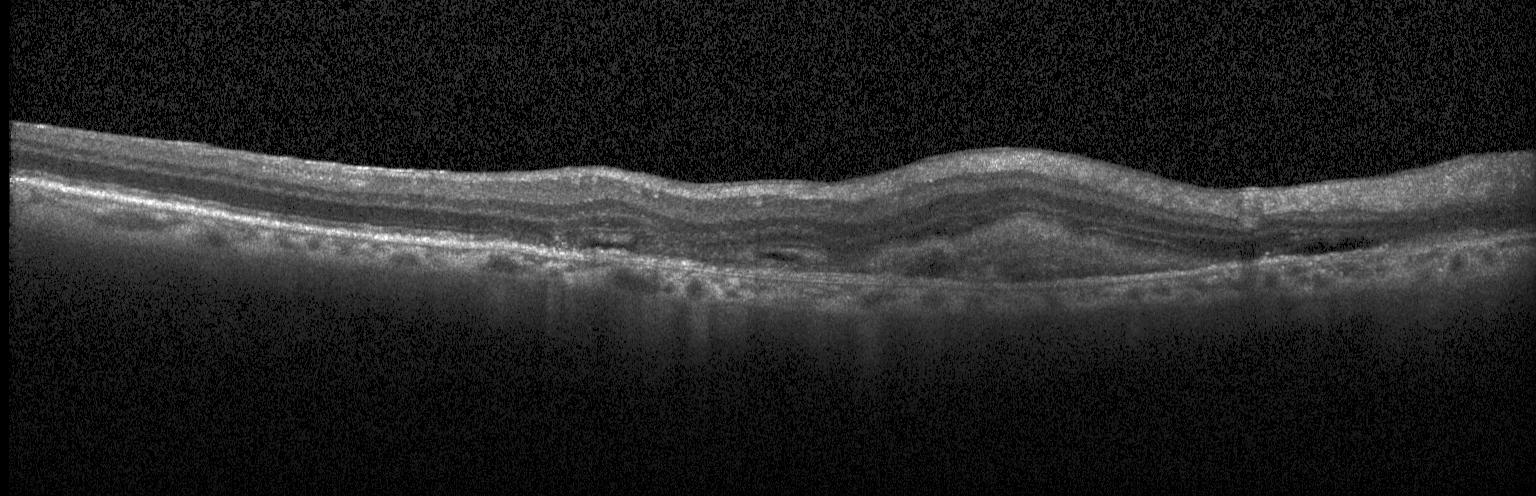

Optical coherence tomography scan; spectral-domain OCT
OCT finding: choroidal neovascularization.